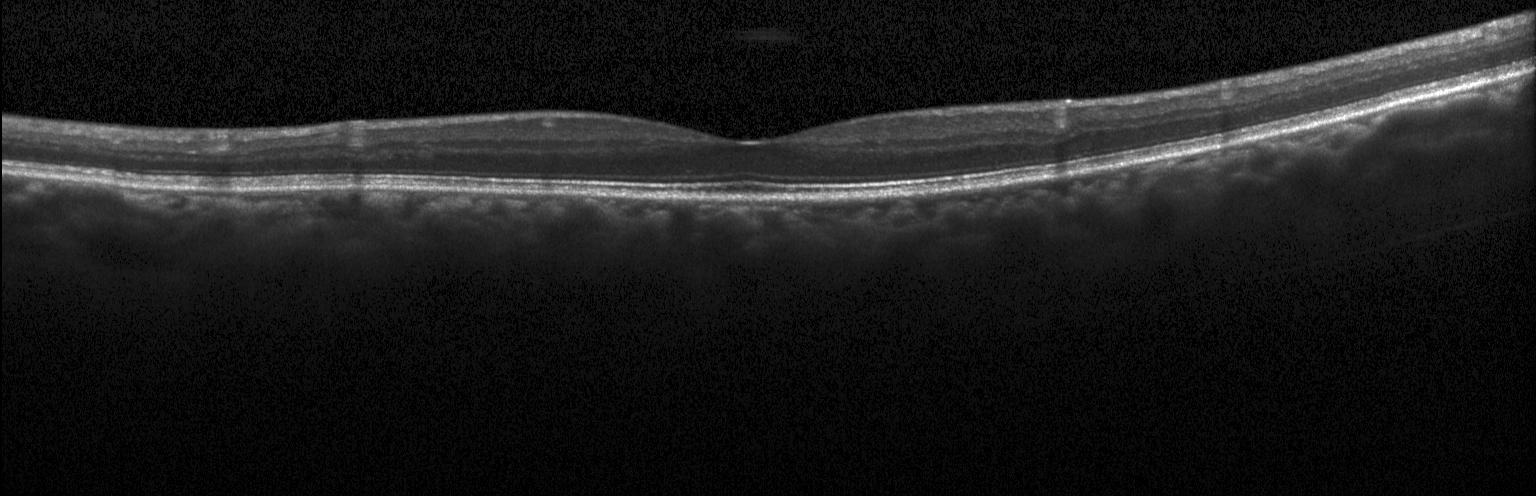

Diagnosis: no choroidal neovascularization, no diabetic macular edema, and no drusen.